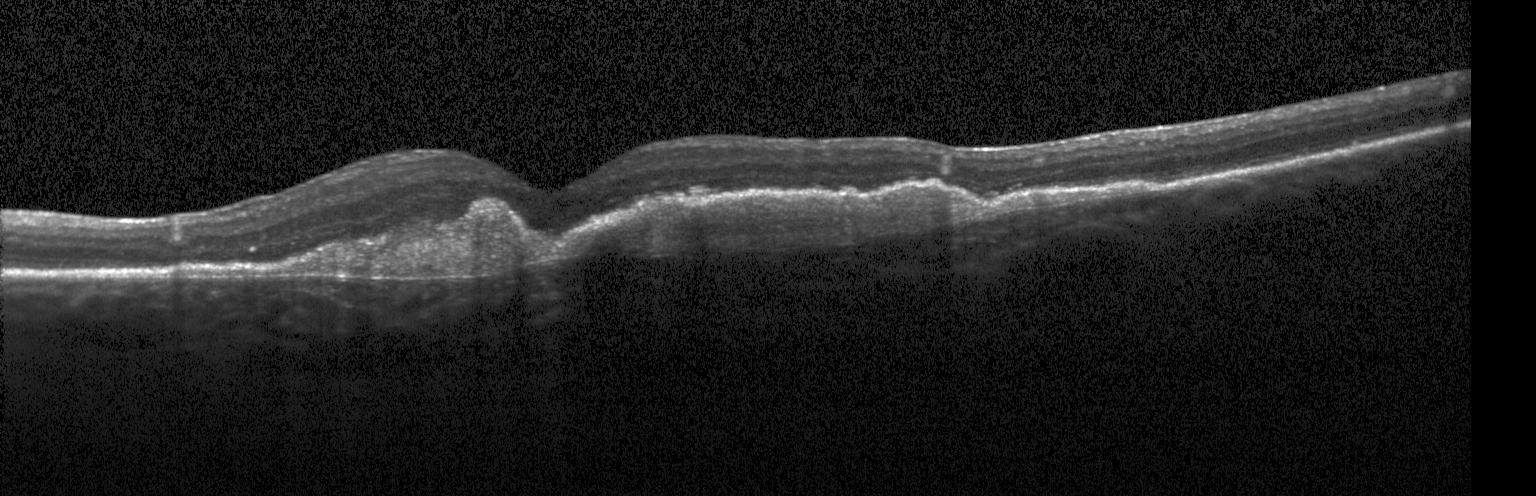
OCT B-scan. Spectral-domain optical coherence tomography. Acquired on a Heidelberg Spectralis. Fovea-centered
Dx: choroidal neovascularization (CNV).